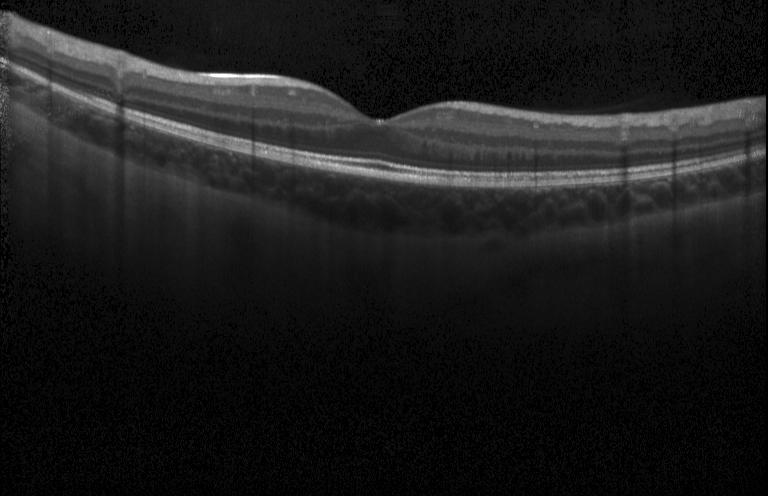 Heidelberg Spectralis OCT system. Retinal OCT cross-section
Finding: no evidence of choroidal neovascularization, diabetic macular edema, or drusen.